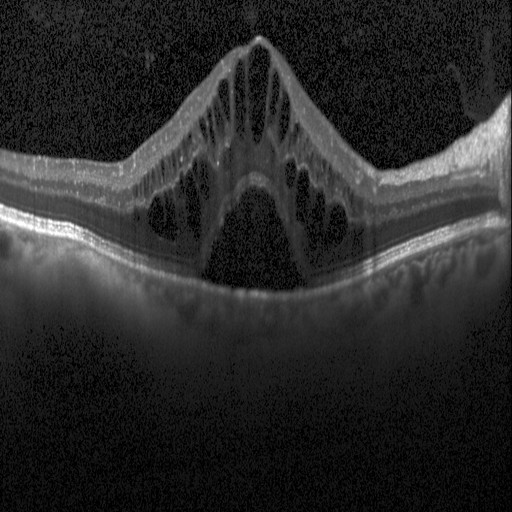

Diabetic macular edema (DME).